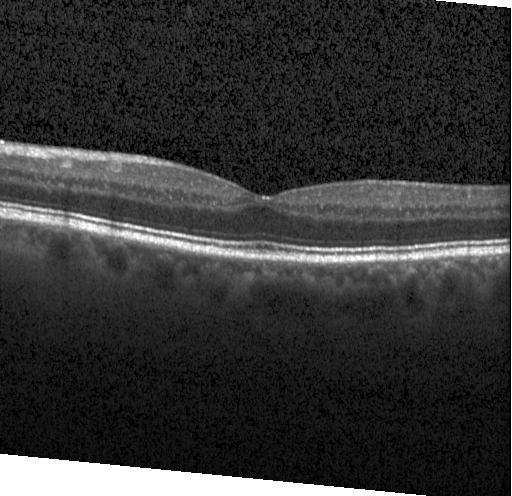

Impression: no evidence of choroidal neovascularization, diabetic macular edema, or drusen.